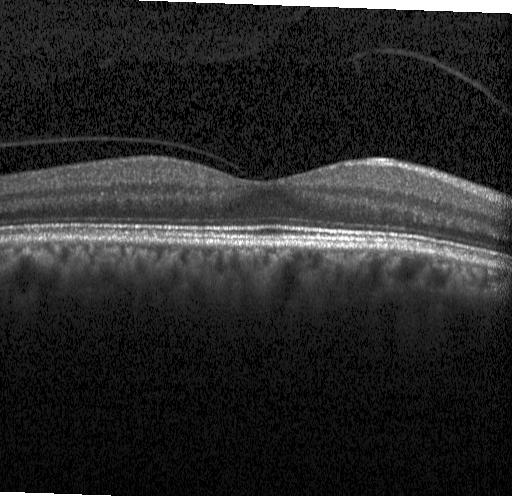 Centered on the fovea · acquired on a Heidelberg Spectralis · spectral-domain OCT · OCT line scan.
This B-scan demonstrates neither choroidal neovascularization, diabetic macular edema, nor drusen.